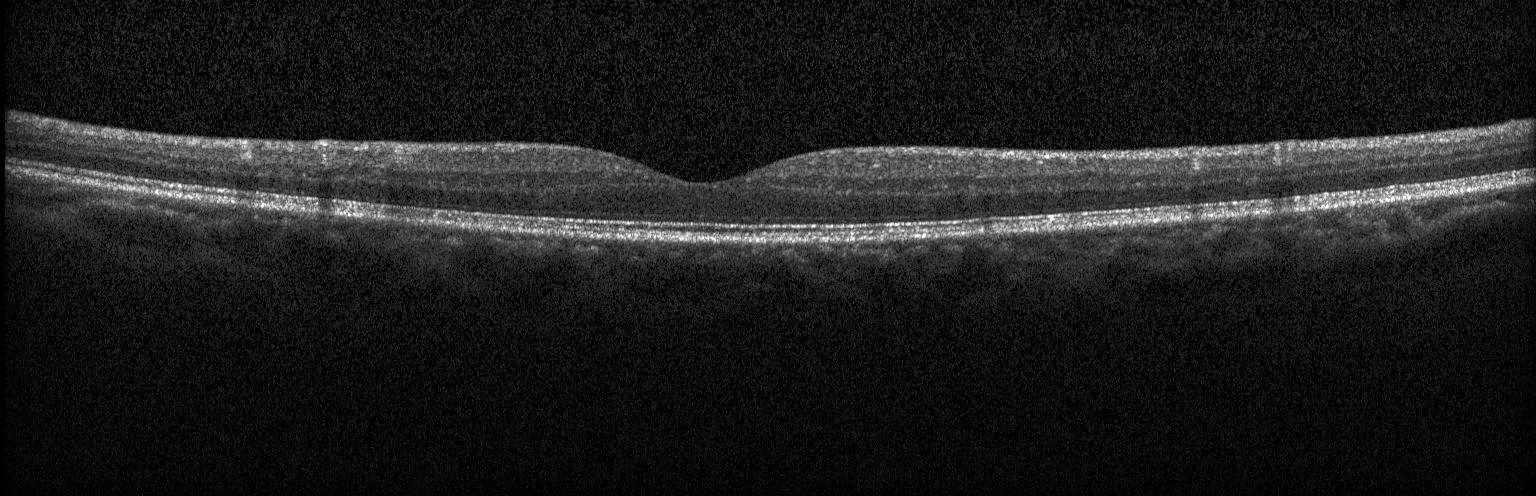

Retinal OCT B-scan. OCT finding: no evidence of choroidal neovascularization, diabetic macular edema, or drusen.